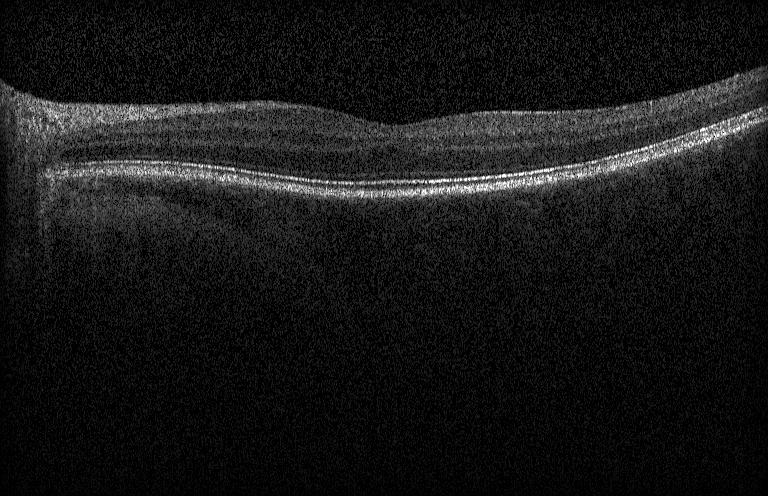
Instrument: Heidelberg Spectralis. OCT B-scan
No CNV, no DME, and no drusen.